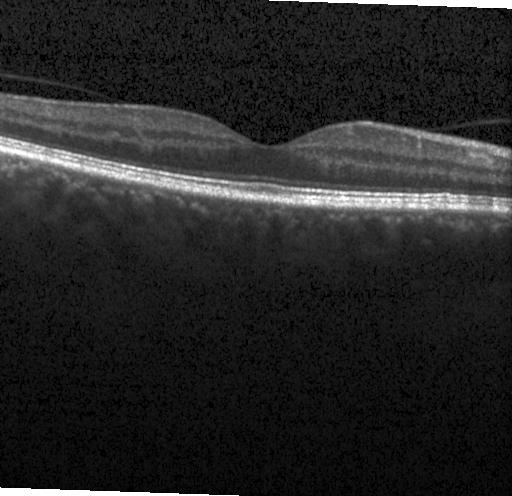

Spectral-domain optical coherence tomography · instrument: Heidelberg Spectralis · optical coherence tomography scan. Assessment: no choroidal neovascularization, diabetic macular edema, or drusen.